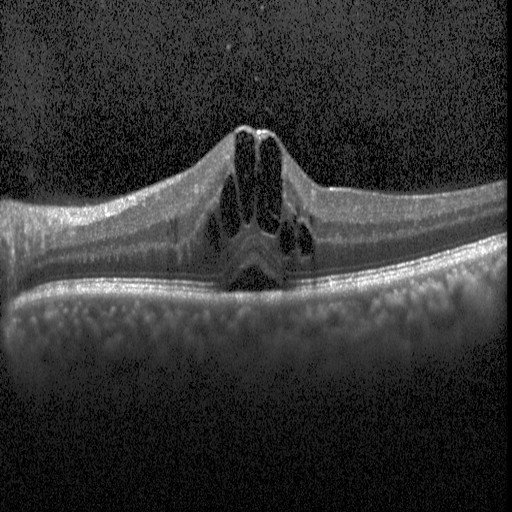 OCT finding: diabetic macular edema (DME).